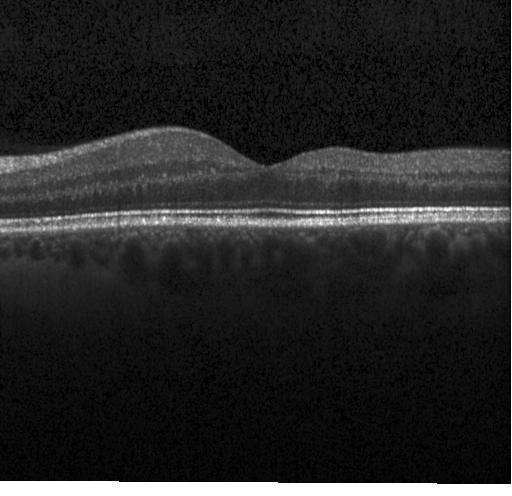 Horizontal scan through the fovea, acquired on a Heidelberg Spectralis, retinal OCT cross-section. Macular OCT: no evidence of choroidal neovascularization, diabetic macular edema, or drusen.